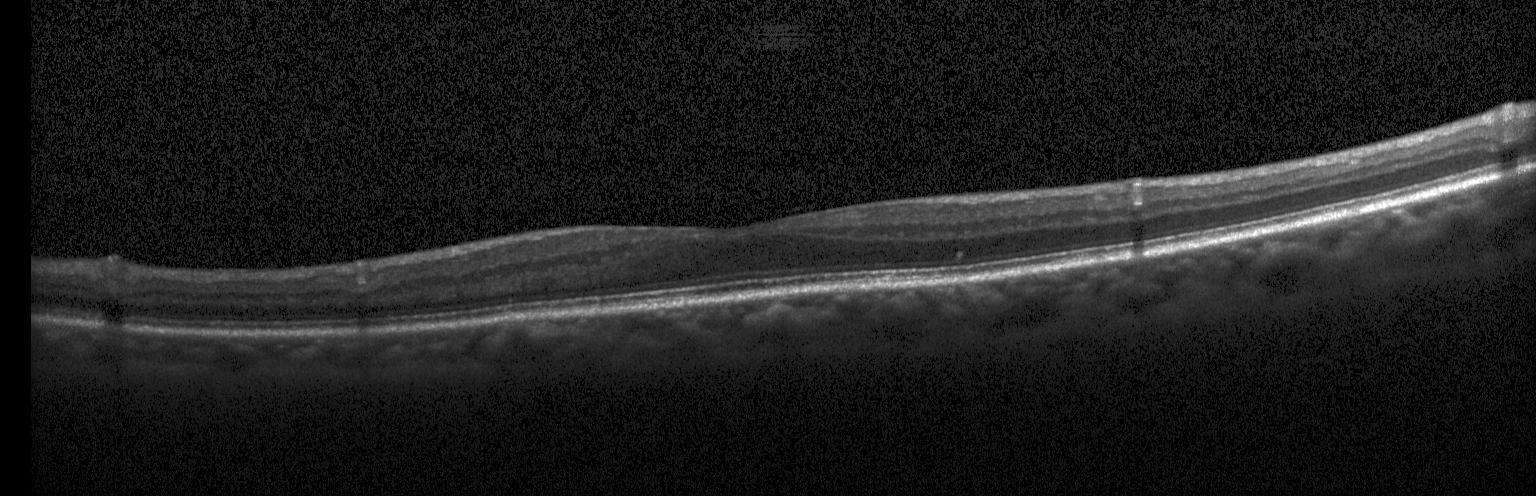 OCT B-scan showing no choroidal neovascularization, no diabetic macular edema, and no drusen.